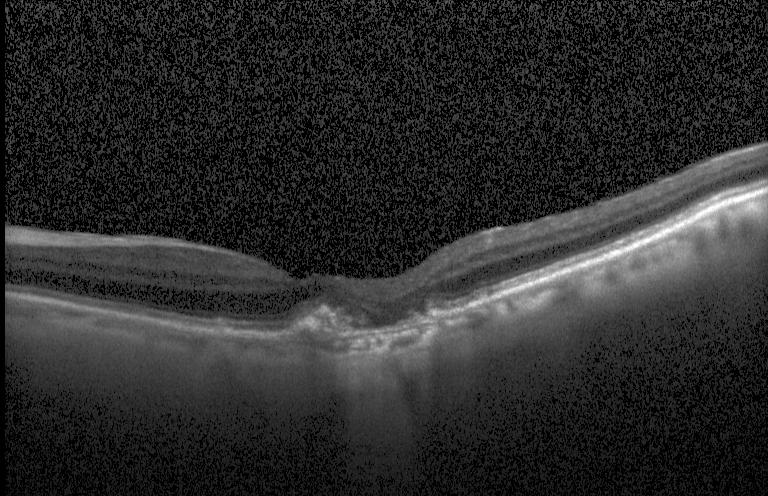
Spectral-domain optical coherence tomography; optical coherence tomography scan
Impression: CNV.